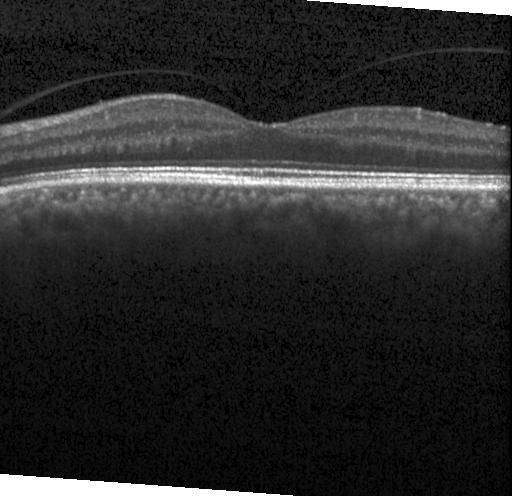
Diagnosis: no choroidal neovascularization, diabetic macular edema, or drusen.